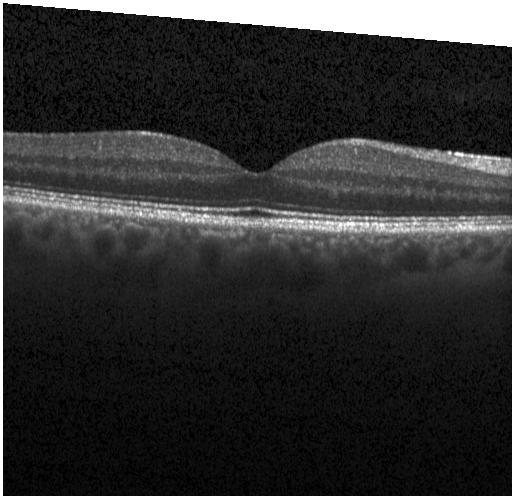
This B-scan demonstrates no choroidal neovascularization, diabetic macular edema, or drusen.